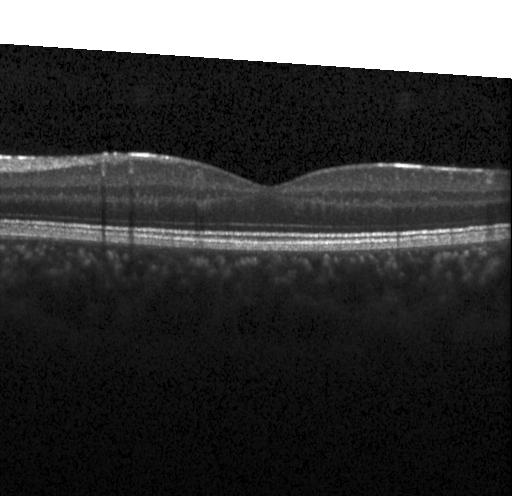 Dx: no evidence of CNV, DME, or drusen.